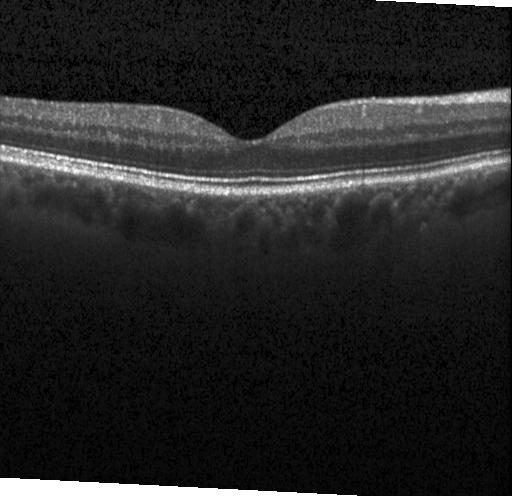
Optical coherence tomography scan; acquired on a Heidelberg Spectralis — Assessment: no evidence of choroidal neovascularization, diabetic macular edema, or drusen.